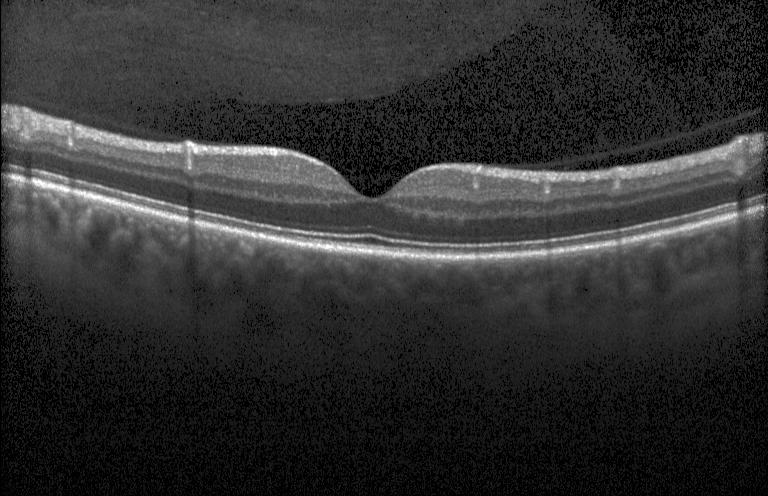

OCT B-scan — Diagnosis: no CNV, DME, or drusen.